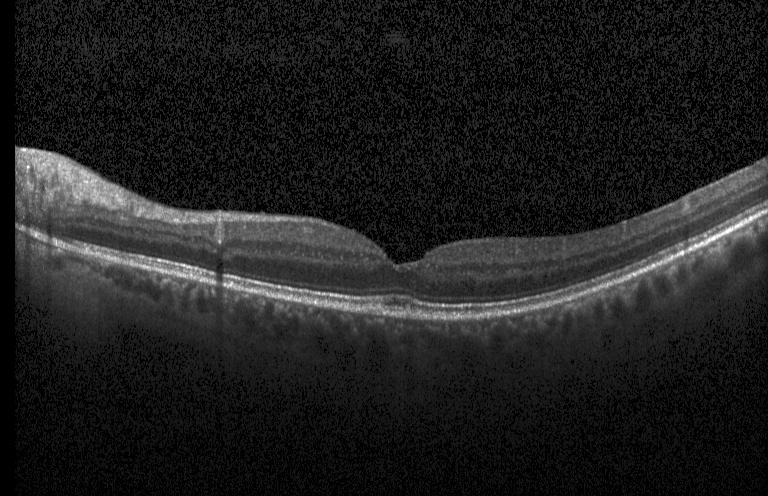
Dx: no evidence of choroidal neovascularization, diabetic macular edema, or drusen.